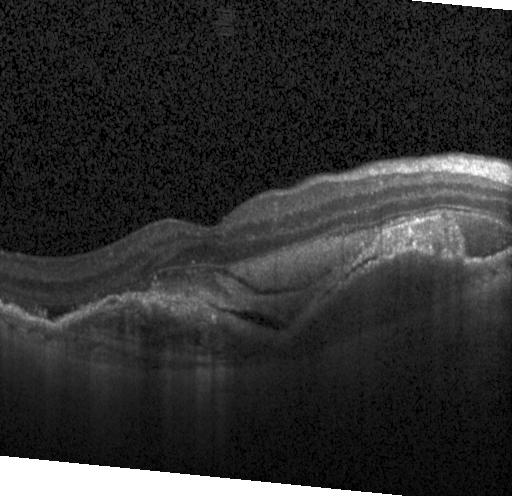 Retinal OCT cross-section. This B-scan demonstrates CNV.